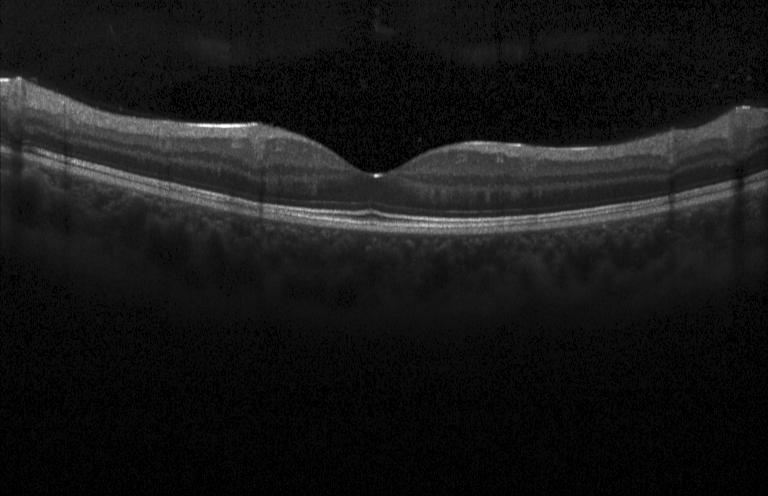

Retinal OCT B-scan — Diagnosis: no evidence of CNV, DME, or drusen.